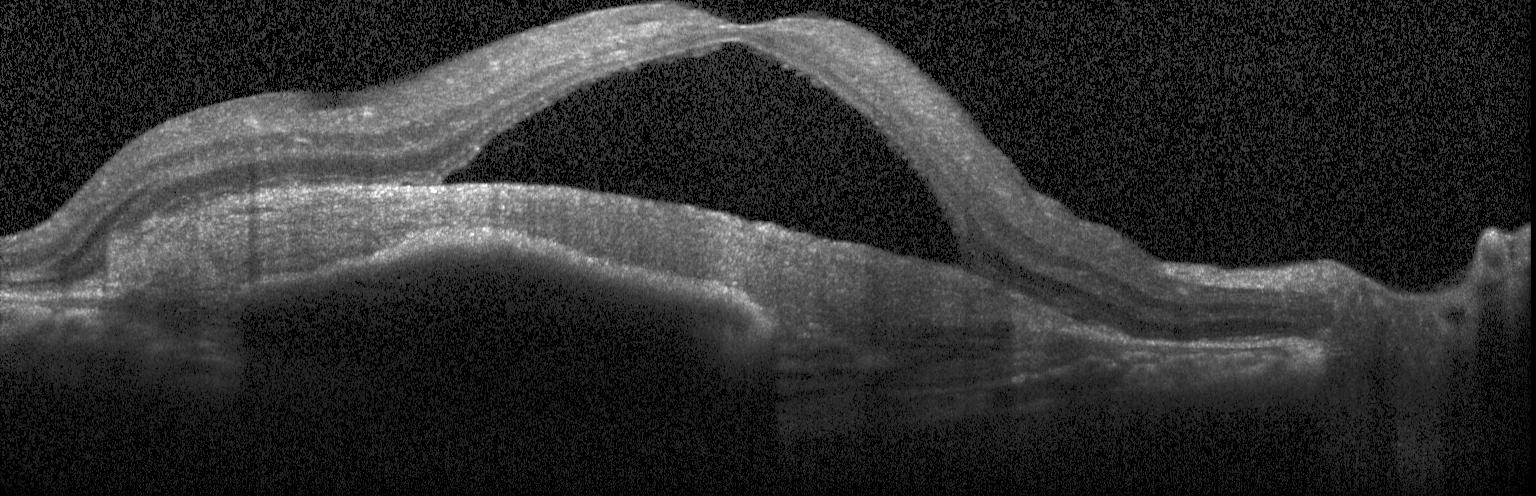
OCT line scan.
Finding: a choroidal neovascular membrane.